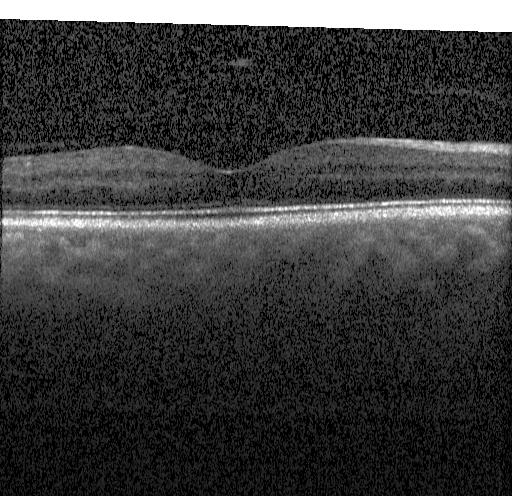
OCT scan showing no choroidal neovascularization, no diabetic macular edema, and no drusen.